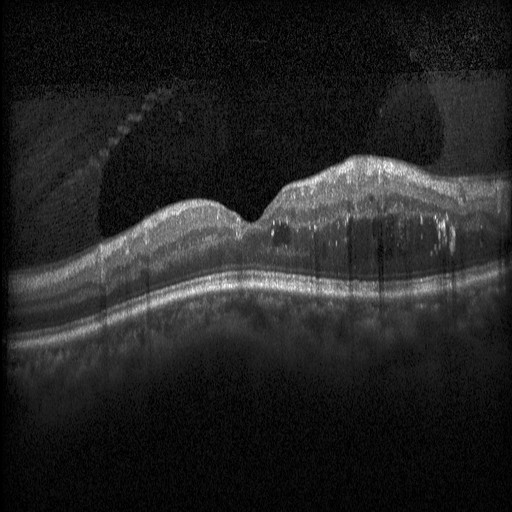
Heidelberg Spectralis OCT system, OCT line scan — Impression: DME.